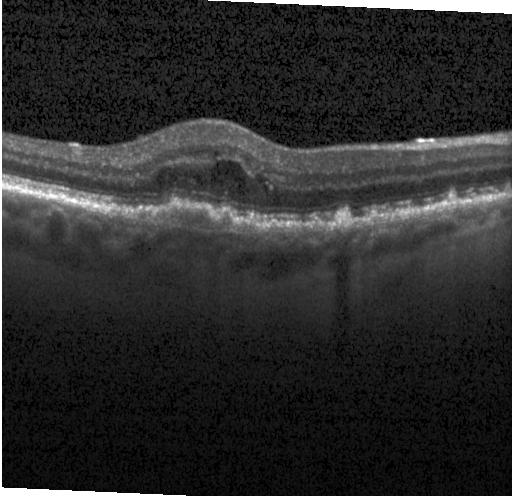 Acquired on a Heidelberg Spectralis; OCT B-scan; SD-OCT — Finding: choroidal neovascularization.